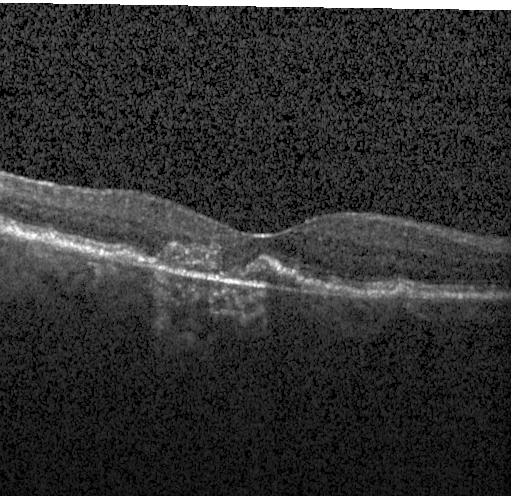

OCT B-scan
A choroidal neovascular membrane.